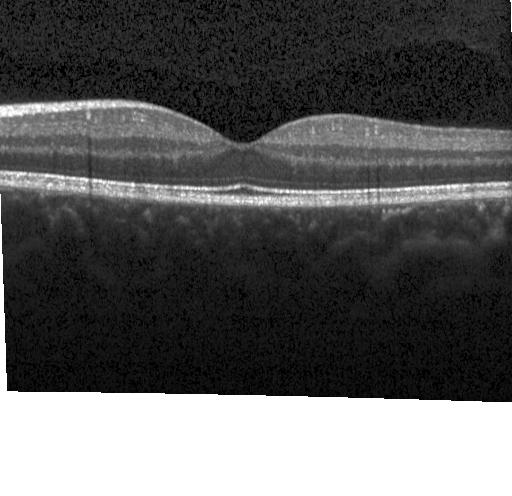
Diagnosis: neither choroidal neovascularization, diabetic macular edema, nor drusen.